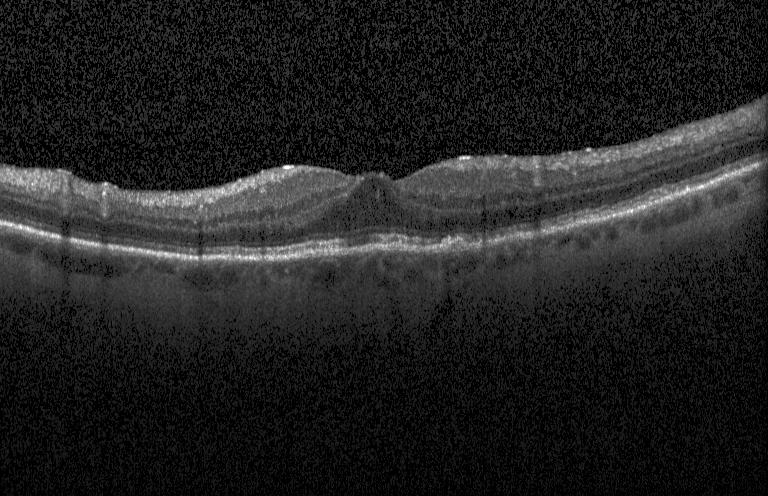 Macular OCT demonstrating drusen.